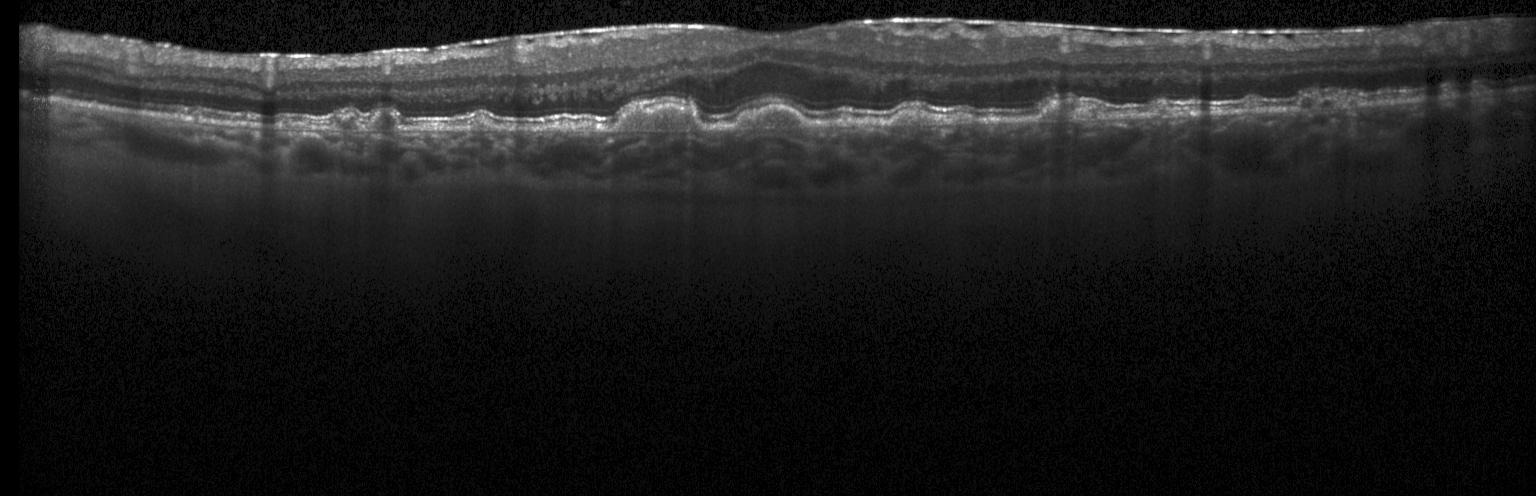 Optical coherence tomography scan, horizontal scan through the fovea, Heidelberg Spectralis OCT system, SD-OCT.
Finding: a choroidal neovascular membrane.